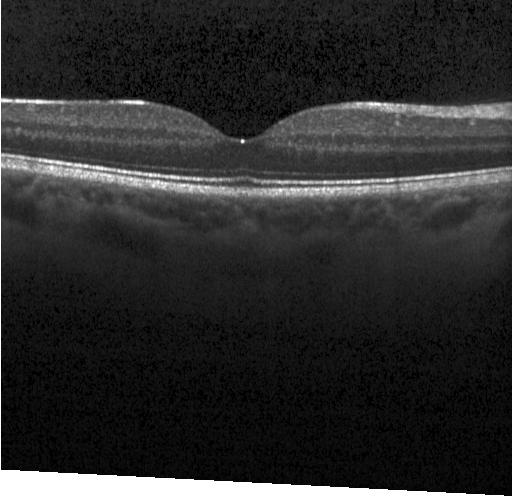

Acquired on a Heidelberg Spectralis, optical coherence tomography scan — Diagnosis: no choroidal neovascularization, no diabetic macular edema, and no drusen.